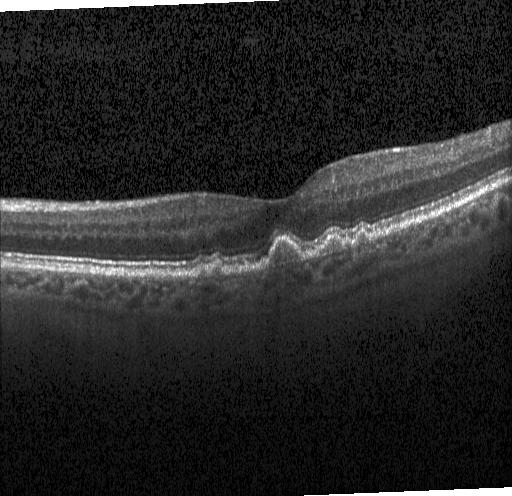
Dx: drusen.